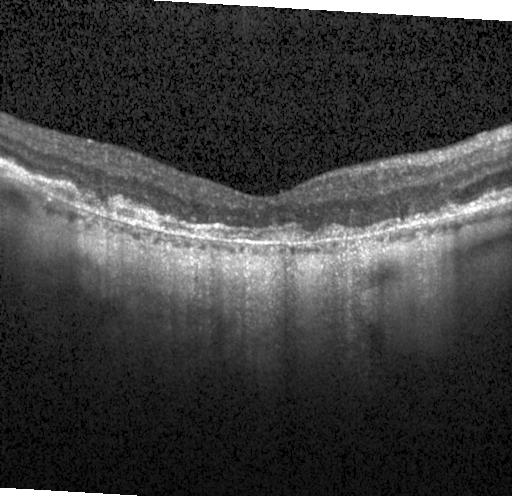 Macular scan · OCT line scan.
A choroidal neovascular membrane.